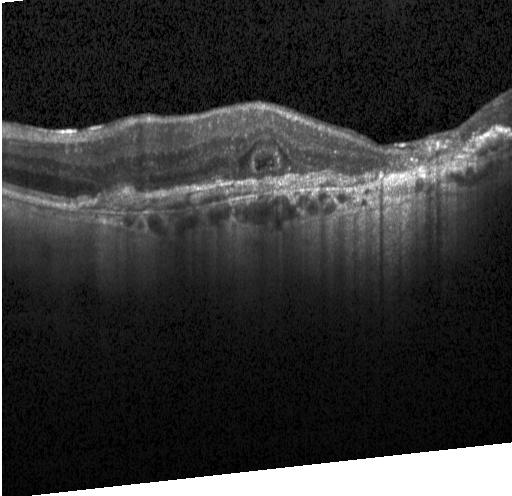 Spectral-domain OCT B-scan: choroidal neovascularization (CNV).